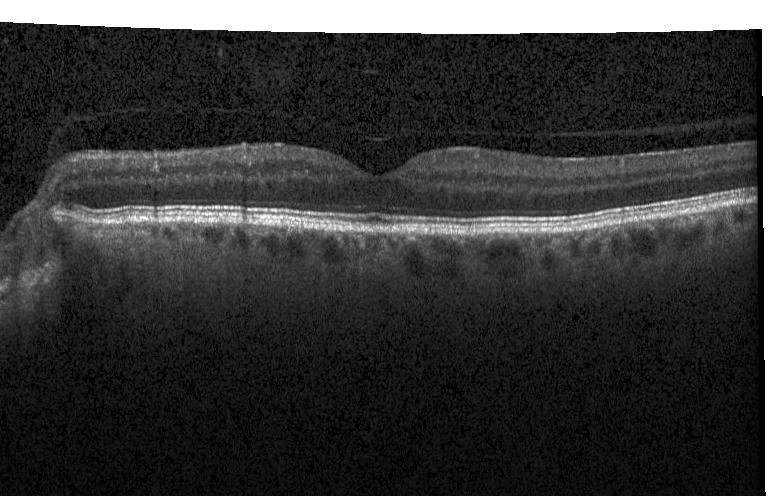
OCT line scan. Centered on the fovea.
Diagnosis: neither choroidal neovascularization, diabetic macular edema, nor drusen.